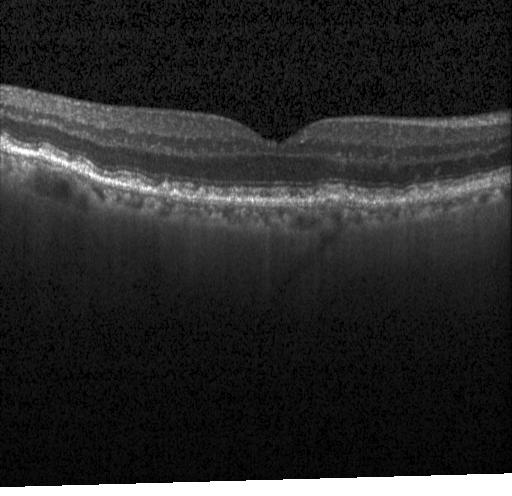 Heidelberg Spectralis OCT system; optical coherence tomography scan; spectral-domain OCT. Finding: sub-RPE drusenoid deposits.